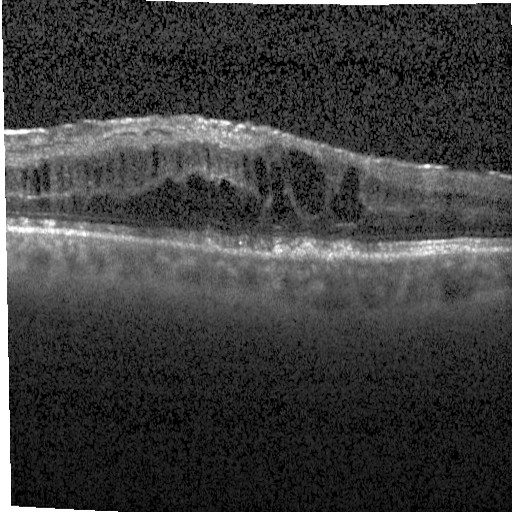

Diabetic macular edema (DME).